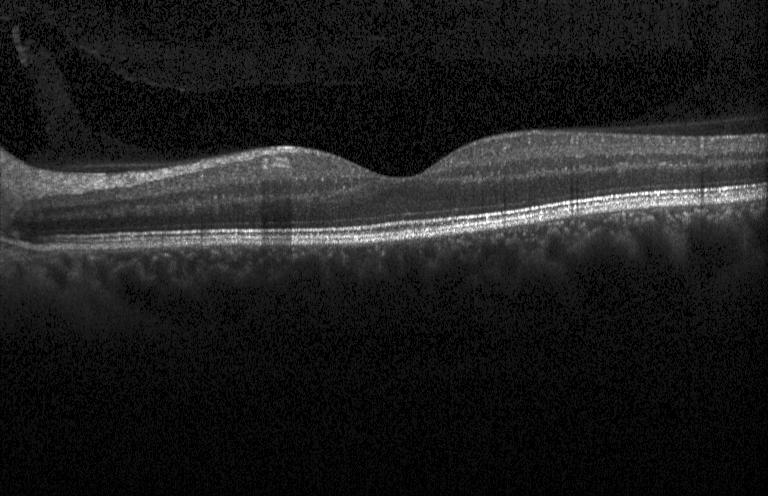 Retinal OCT cross-section. Assessment: no choroidal neovascularization, diabetic macular edema, or drusen.